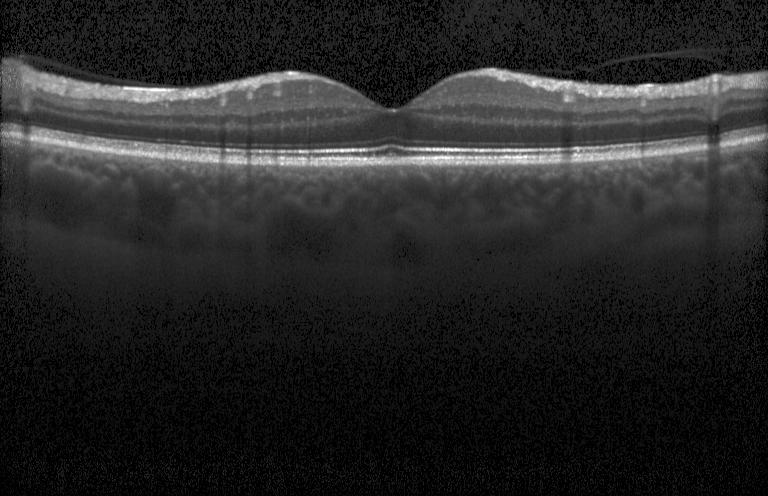

Retinal OCT cross-section showing neither choroidal neovascularization, diabetic macular edema, nor drusen.